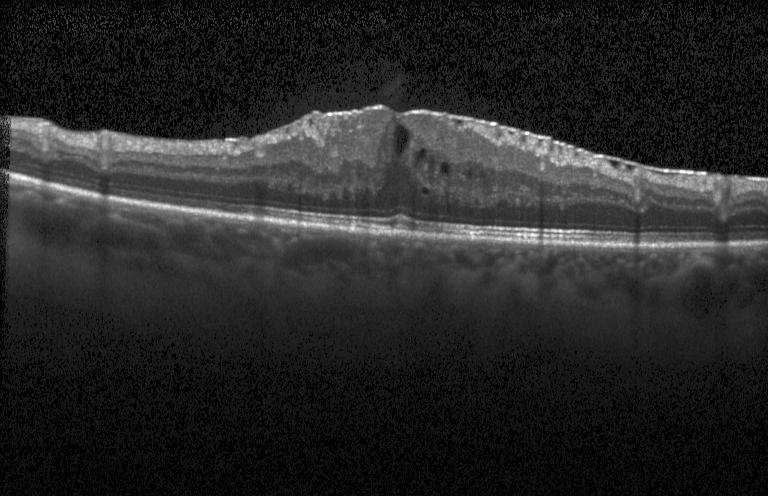

Horizontal scan through the fovea, optical coherence tomography scan. Dx: diabetic macular edema (DME).